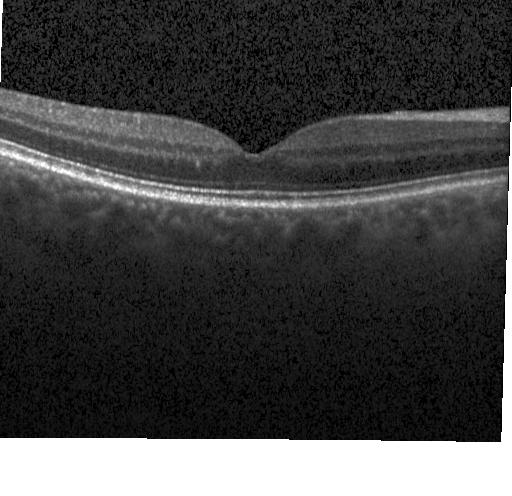 Fovea-centered. Optical coherence tomography scan. Spectral-domain optical coherence tomography. Diagnosis: neither CNV, DME, nor drusen.